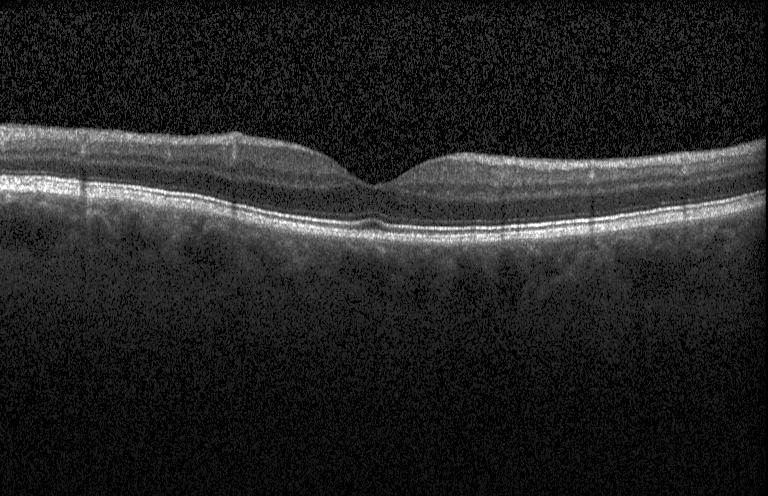 Impression: no choroidal neovascularization, diabetic macular edema, or drusen.